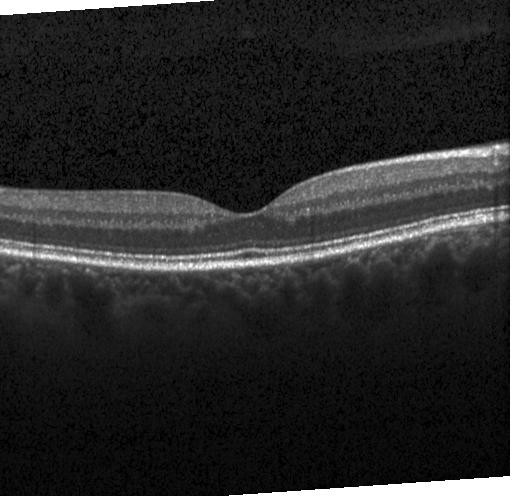 Heidelberg Spectralis; retinal OCT B-scan; SD-OCT; horizontal scan through the fovea. The scan shows neither choroidal neovascularization, diabetic macular edema, nor drusen.